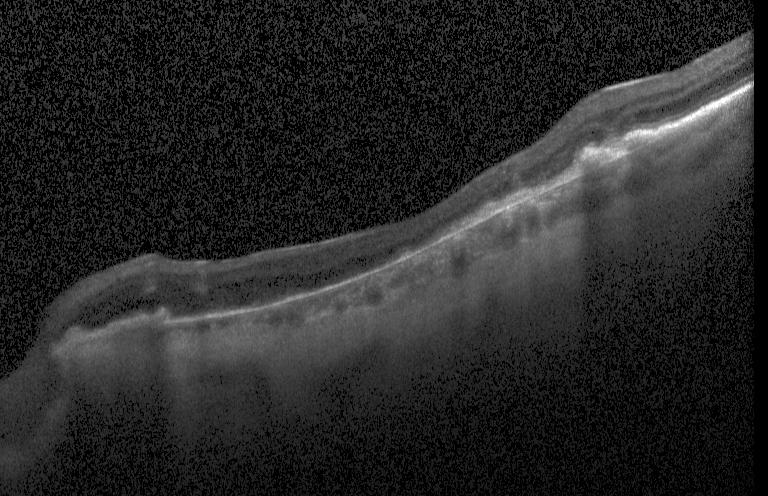
Instrument: Heidelberg Spectralis · retinal OCT cross-section.
Assessment: choroidal neovascularization (CNV).